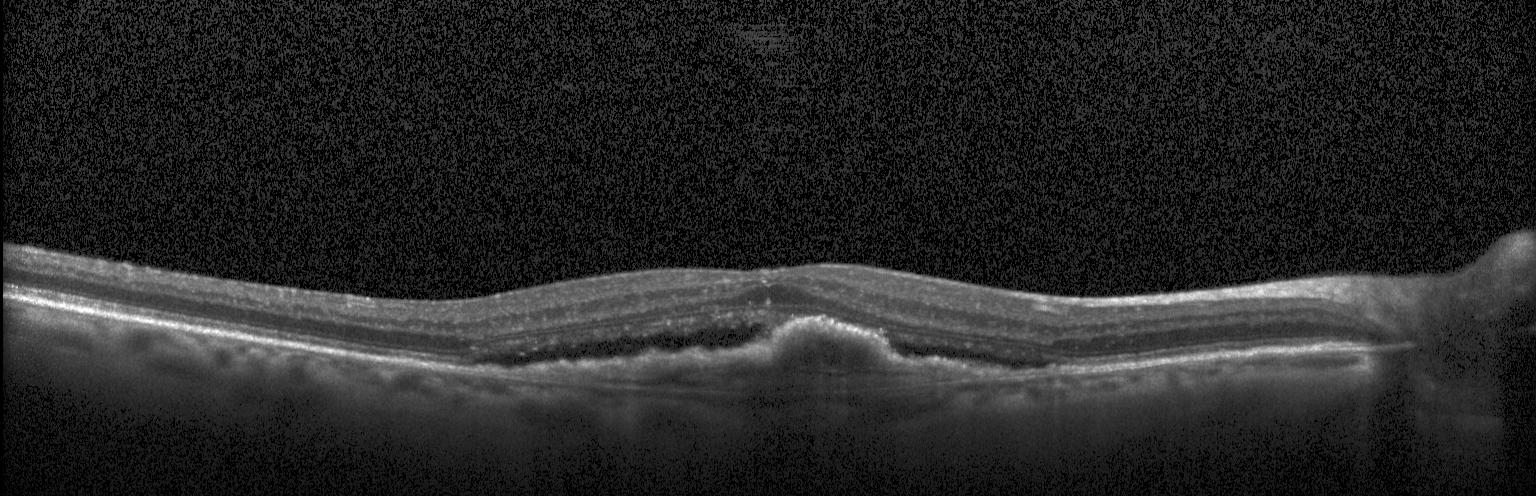 OCT line scan.
This B-scan demonstrates a choroidal neovascular membrane.